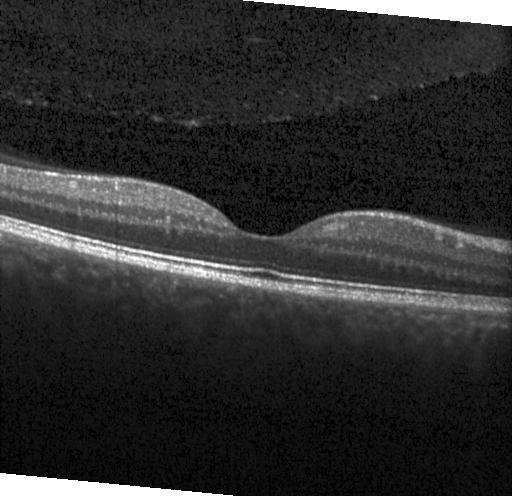
Diagnosis: neither CNV, DME, nor drusen.